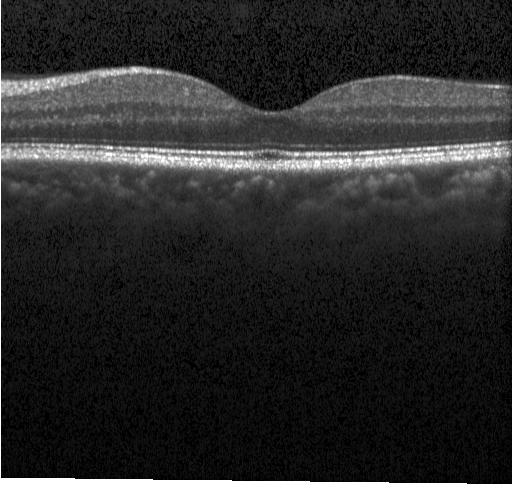 Heidelberg Spectralis OCT system; spectral-domain OCT; retinal OCT B-scan; through the macula — This B-scan demonstrates no choroidal neovascularization, diabetic macular edema, or drusen.